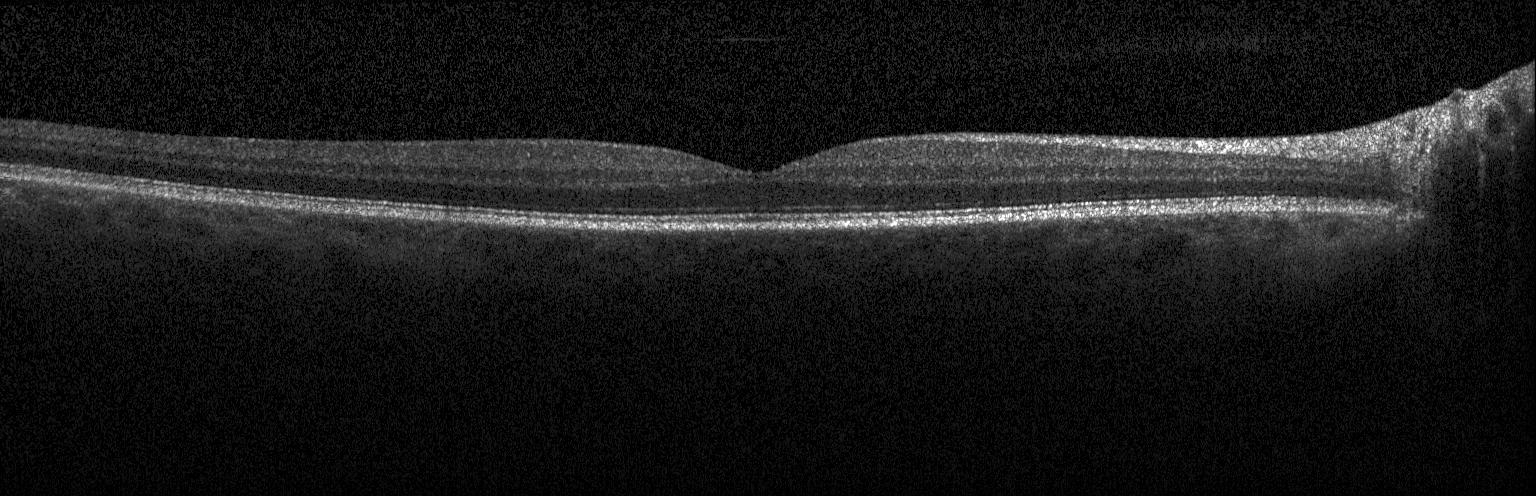 The scan shows neither CNV, DME, nor drusen.